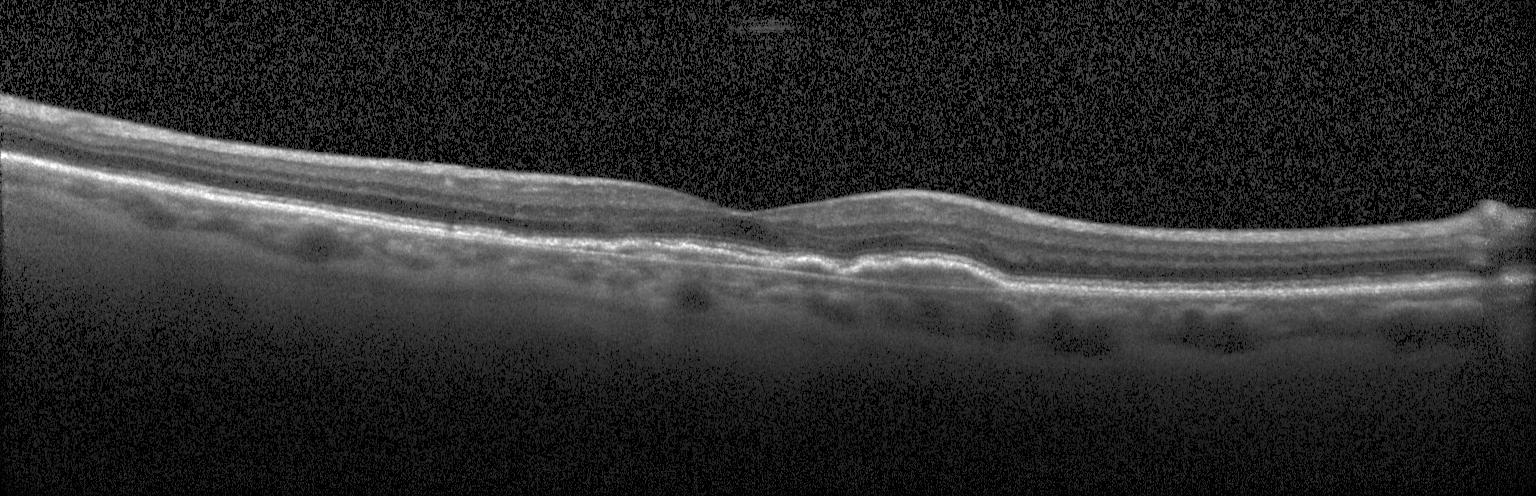
Optical coherence tomography B-scan · instrument: Heidelberg Spectralis · spectral-domain optical coherence tomography · centered on the fovea.
Assessment: a choroidal neovascular membrane.